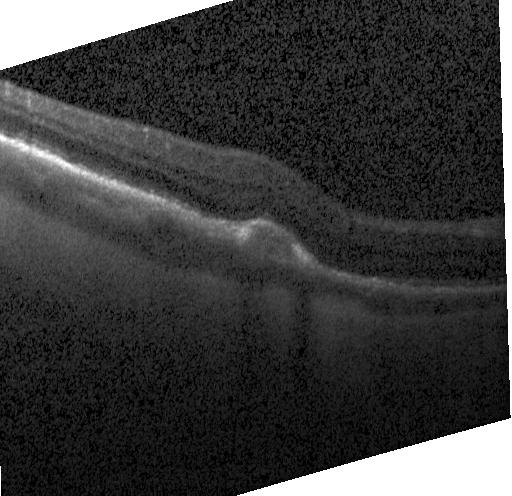

Optical coherence tomography scan · spectral-domain optical coherence tomography · through the macula — Impression: a choroidal neovascular membrane.